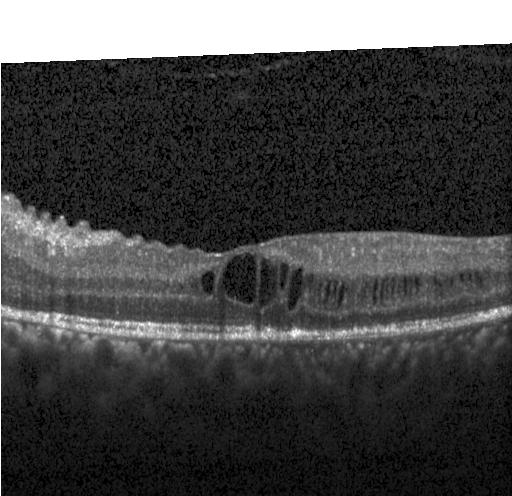 Instrument: Heidelberg Spectralis. OCT B-scan. Impression: diabetic macular edema (DME).